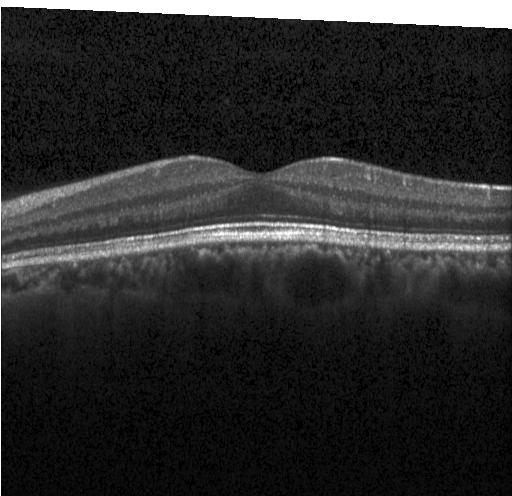
Acquired on a Heidelberg Spectralis. OCT B-scan. This B-scan demonstrates no choroidal neovascularization, no diabetic macular edema, and no drusen.